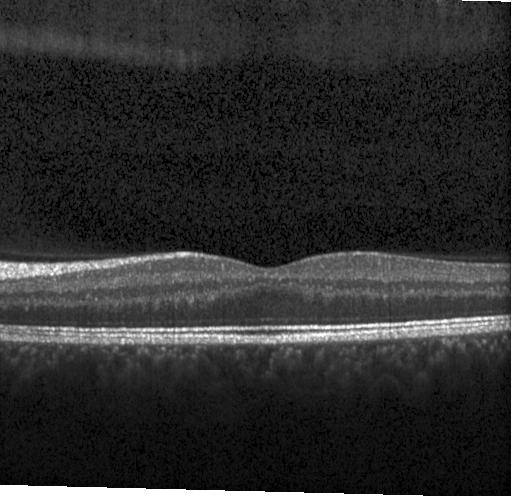 Macular OCT demonstrating neither choroidal neovascularization, diabetic macular edema, nor drusen.